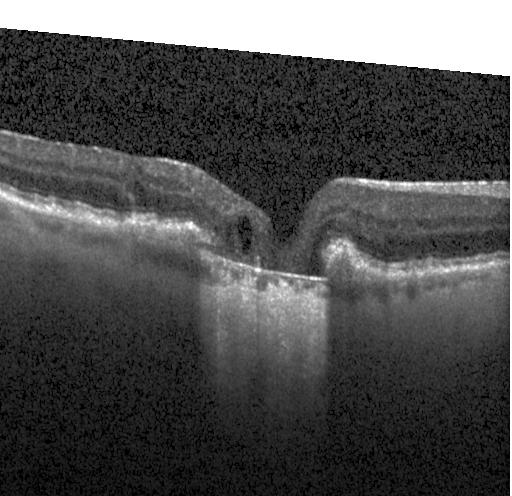
OCT finding: a choroidal neovascular membrane.